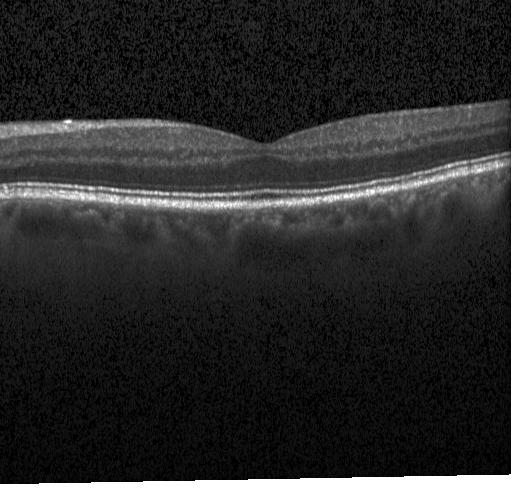
Optical coherence tomography scan — Dx: no evidence of choroidal neovascularization, diabetic macular edema, or drusen.